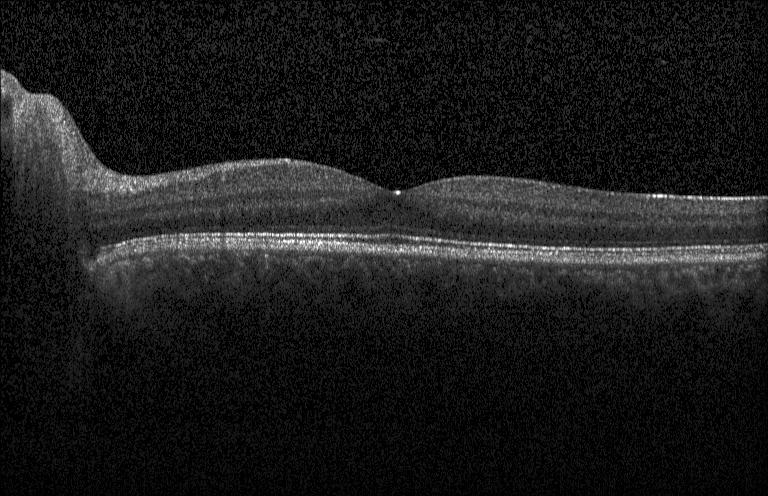 Retinal OCT B-scan. Macular OCT: no choroidal neovascularization, diabetic macular edema, or drusen.